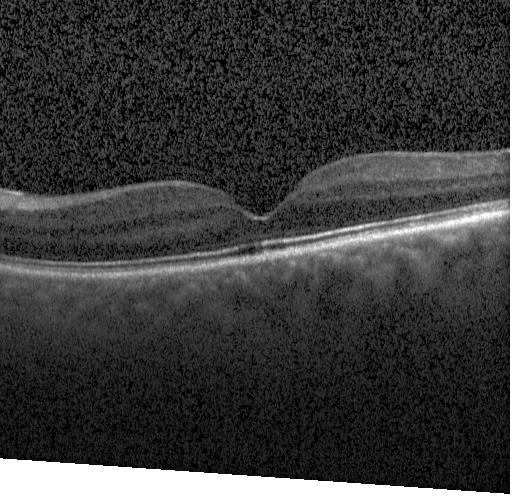

Assessment: no CNV, no DME, and no drusen.